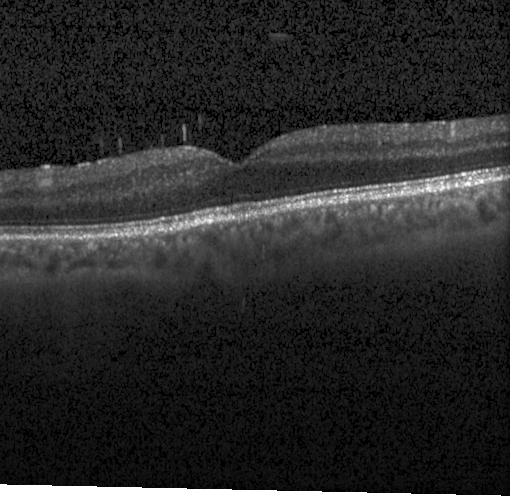 Finding: no evidence of CNV, DME, or drusen.